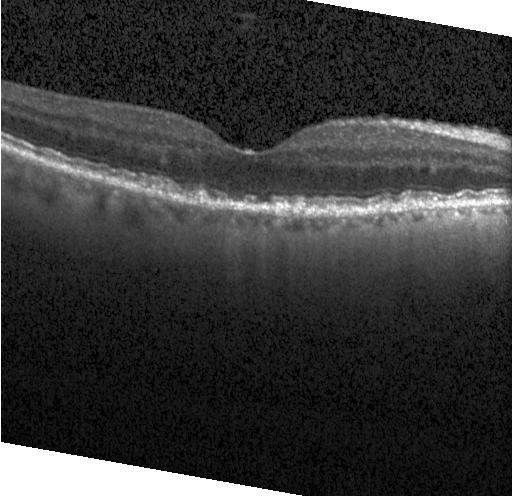 Heidelberg Spectralis · spectral-domain optical coherence tomography · optical coherence tomography B-scan. Finding: sub-RPE drusenoid deposits.